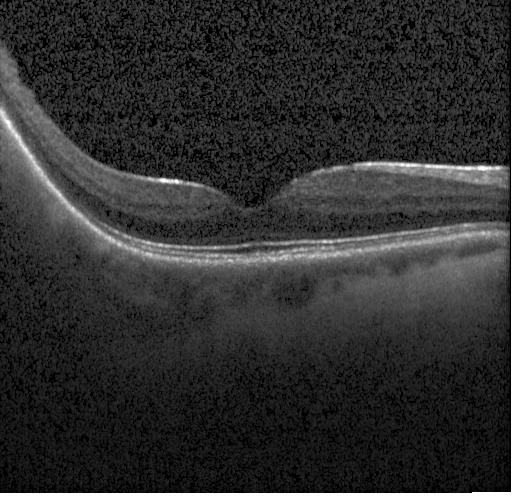 Retinal OCT cross-section showing no evidence of choroidal neovascularization, diabetic macular edema, or drusen.